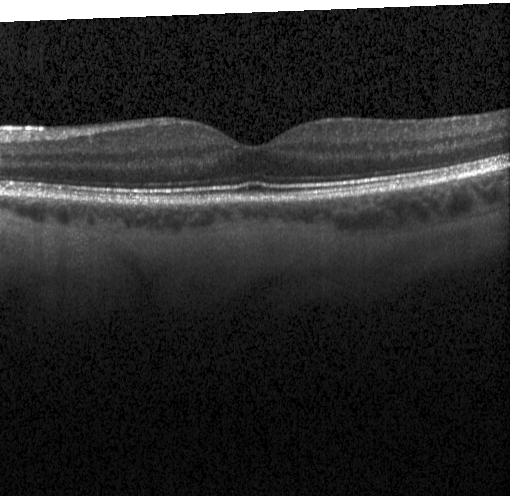

Optical coherence tomography B-scan · spectral-domain OCT.
Impression: neither choroidal neovascularization, diabetic macular edema, nor drusen.